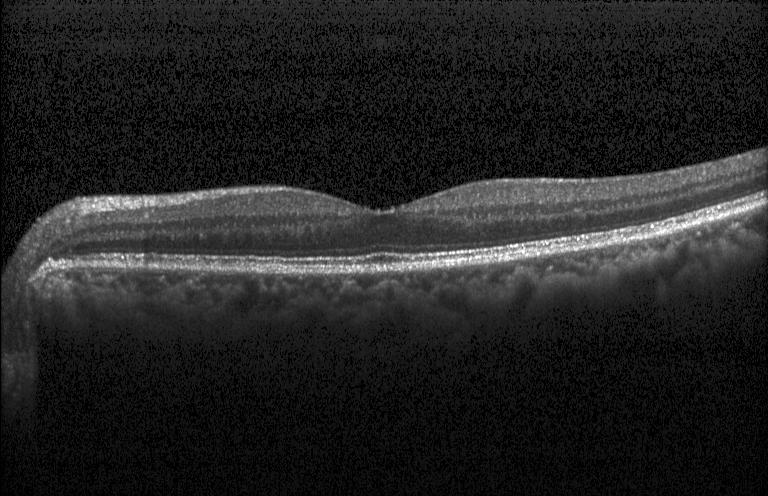
Retinal OCT B-scan.
The scan shows neither choroidal neovascularization, diabetic macular edema, nor drusen.